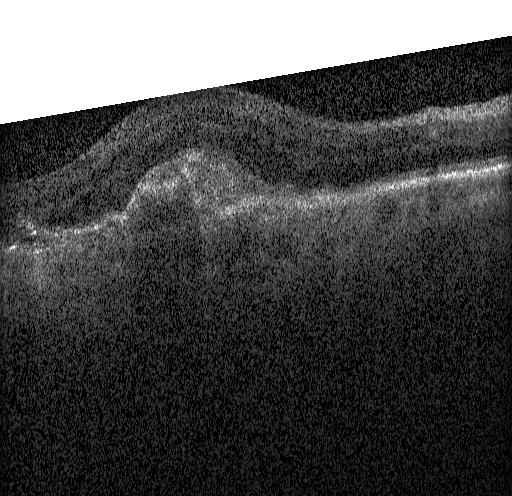
OCT B-scan
Finding: a choroidal neovascular membrane.